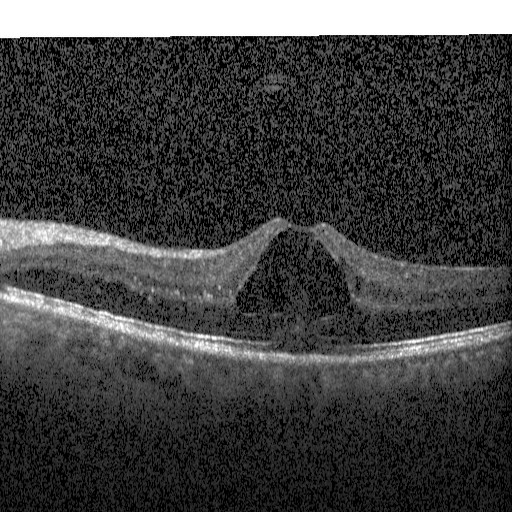

Macular OCT: DME.